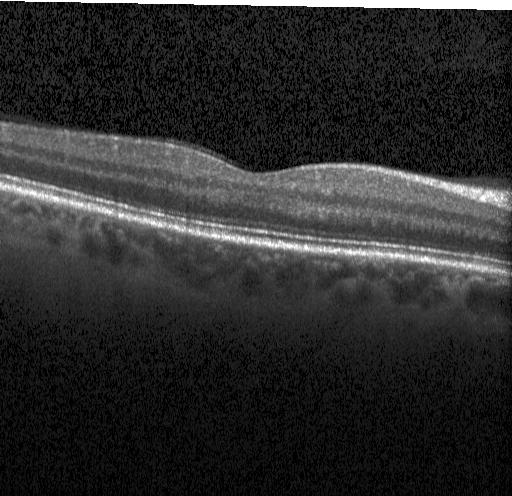 Retinal OCT cross-section.
Dx: no CNV, DME, or drusen.